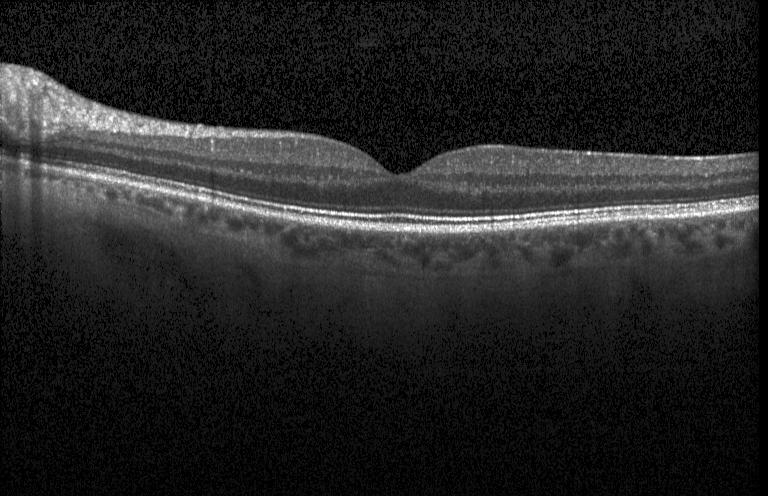

Instrument: Heidelberg Spectralis, spectral-domain optical coherence tomography, retinal OCT cross-section, through the macula
No choroidal neovascularization, diabetic macular edema, or drusen.